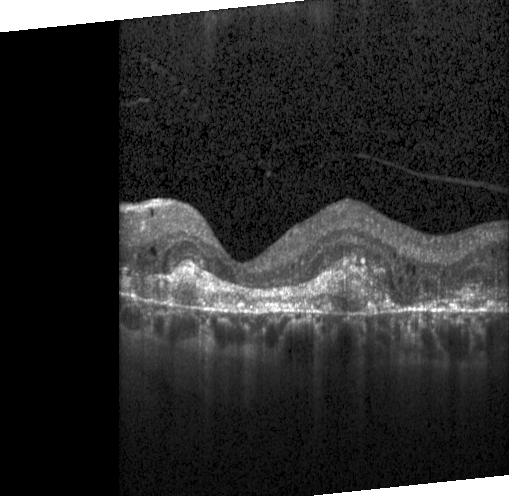

This B-scan demonstrates CNV.